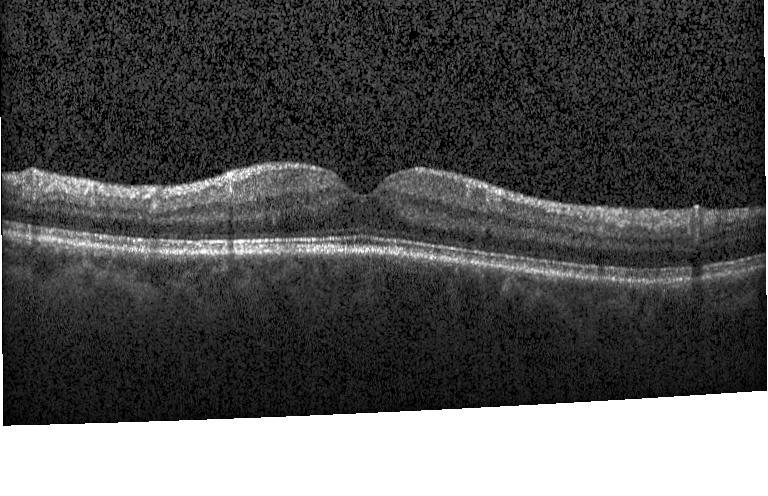
Retinal OCT B-scan. Finding: no choroidal neovascularization, no diabetic macular edema, and no drusen.